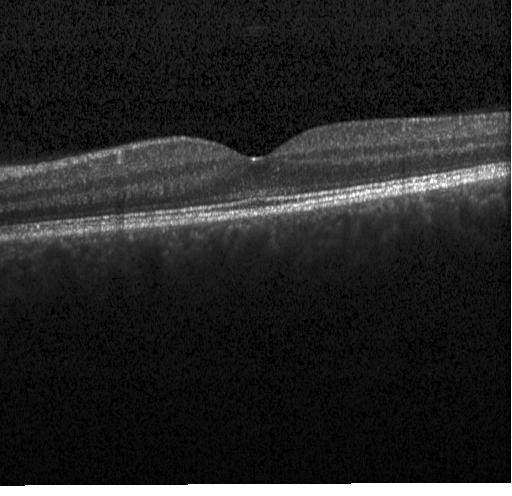

This B-scan demonstrates no choroidal neovascularization, no diabetic macular edema, and no drusen.